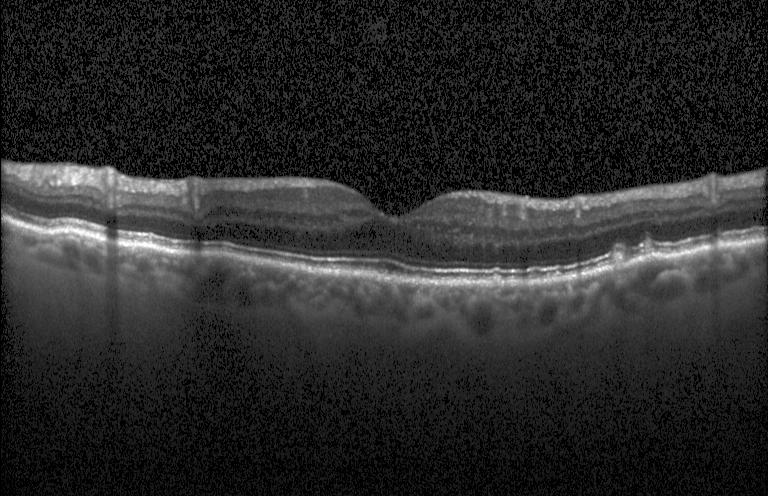 OCT B-scan. Assessment: sub-RPE drusenoid deposits.